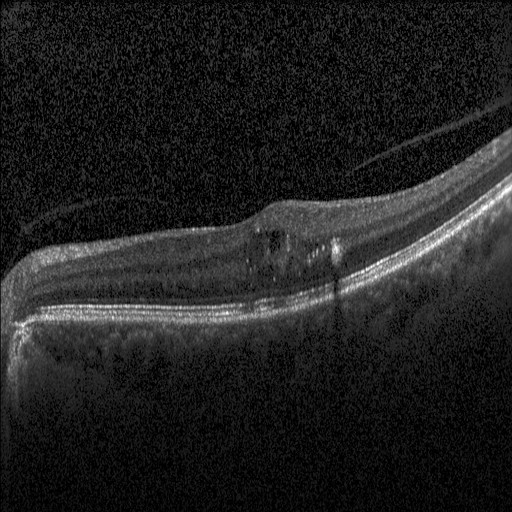
Spectral-domain OCT B-scan: diabetic macular edema.